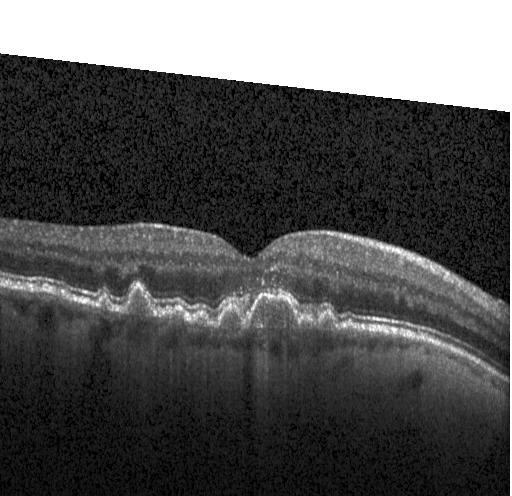
OCT B-scan; horizontal scan through the fovea — The scan shows multiple drusen.